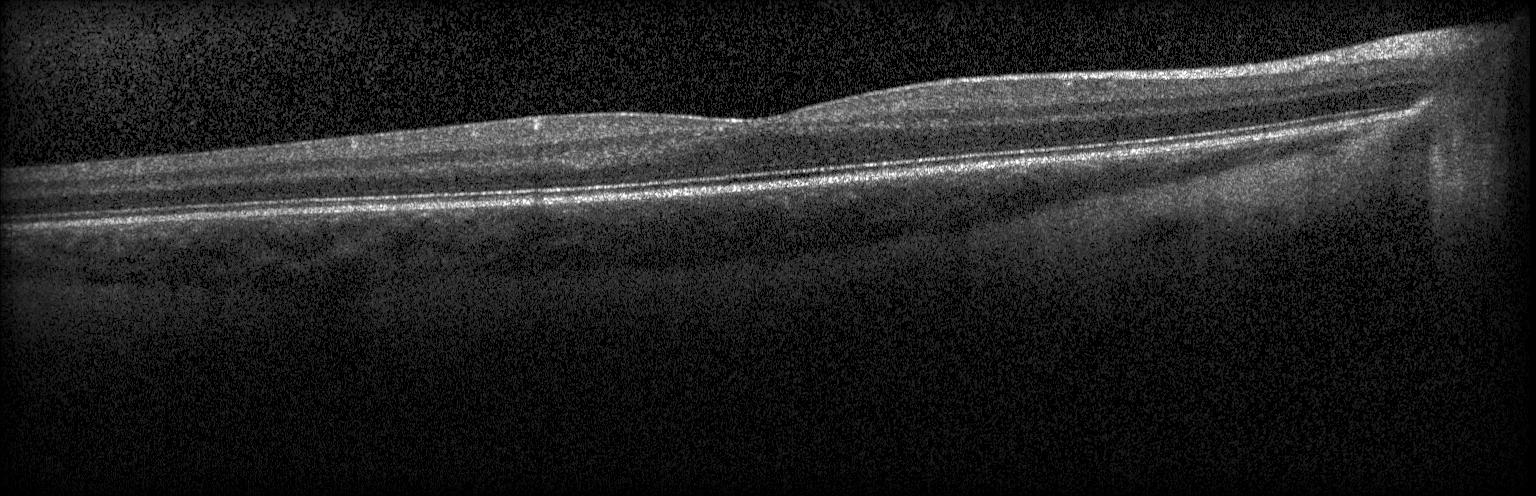

Spectral-domain OCT B-scan: no CNV, DME, or drusen.